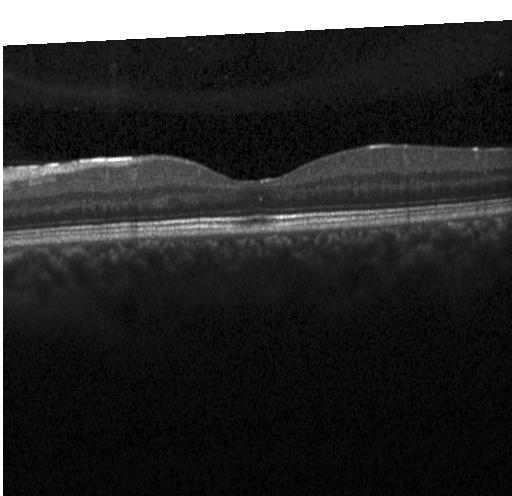
The scan shows neither CNV, DME, nor drusen.